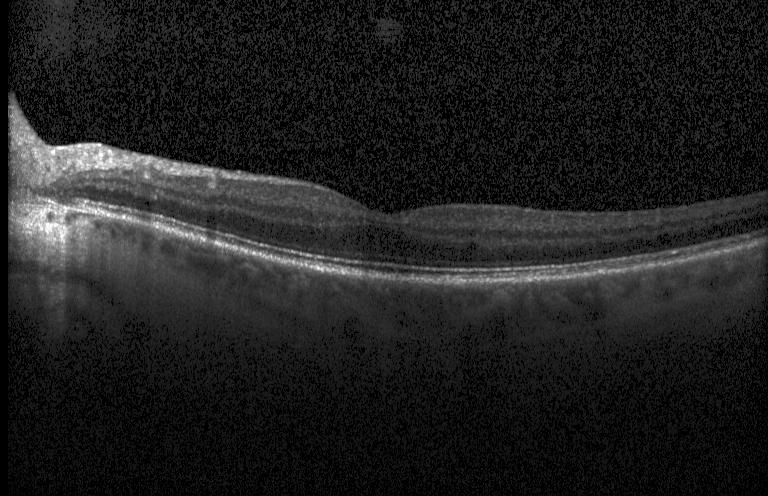
OCT line scan, Heidelberg Spectralis, SD-OCT
This B-scan demonstrates no choroidal neovascularization, diabetic macular edema, or drusen.